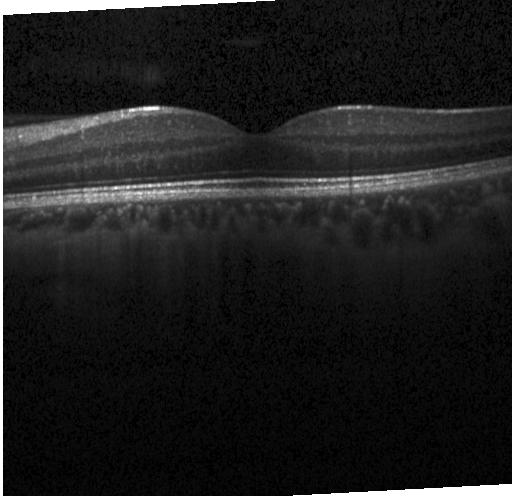

Optical coherence tomography B-scan; spectral-domain optical coherence tomography; through the macula; Heidelberg Spectralis — Impression: no evidence of CNV, DME, or drusen.